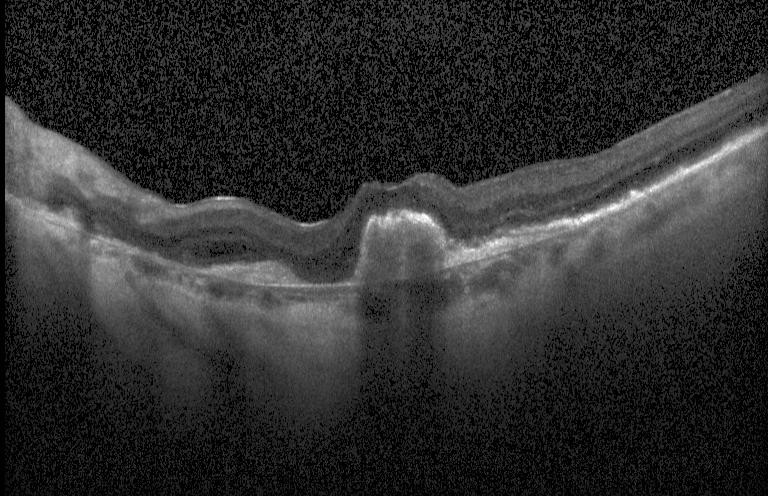 OCT line scan. Assessment: choroidal neovascularization (CNV).